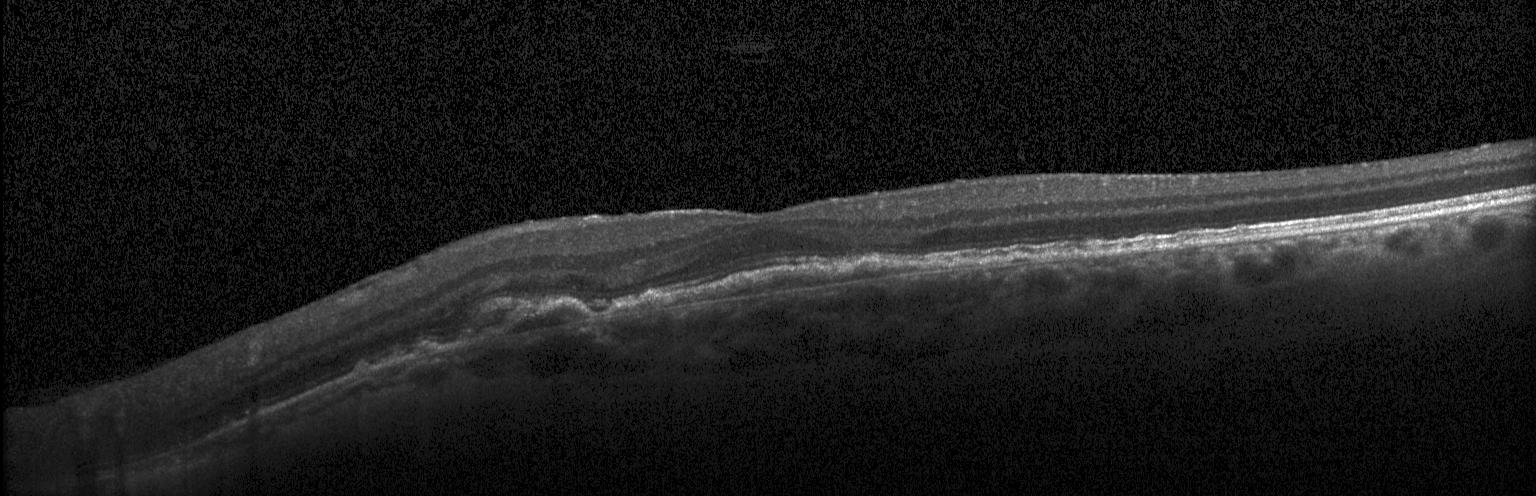
This B-scan demonstrates a choroidal neovascular membrane.